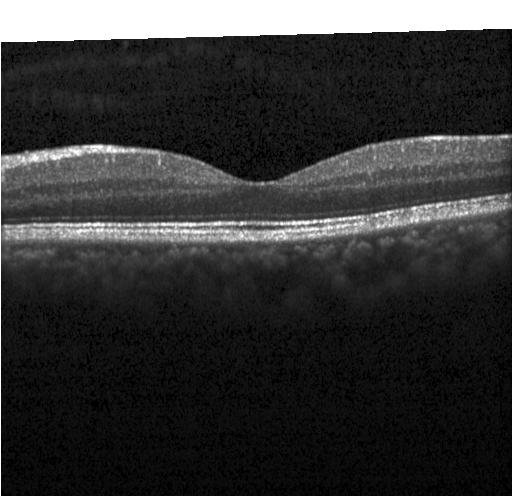 OCT B-scan — No evidence of CNV, DME, or drusen.